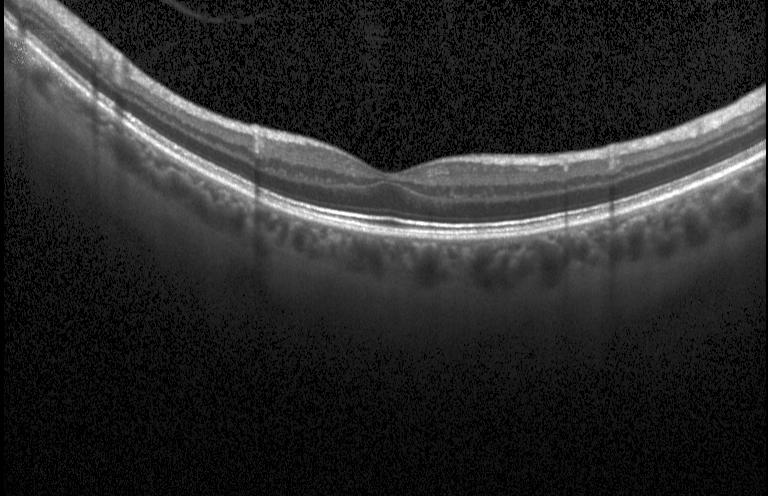

OCT B-scan — Impression: no choroidal neovascularization, diabetic macular edema, or drusen.